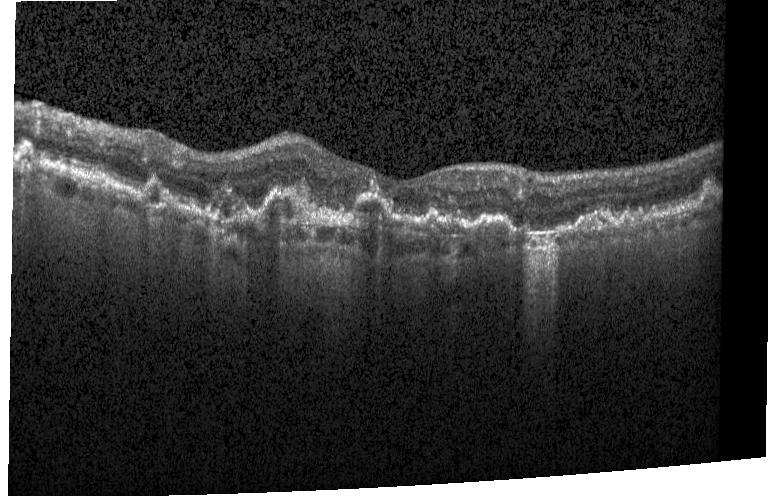
A choroidal neovascular membrane.